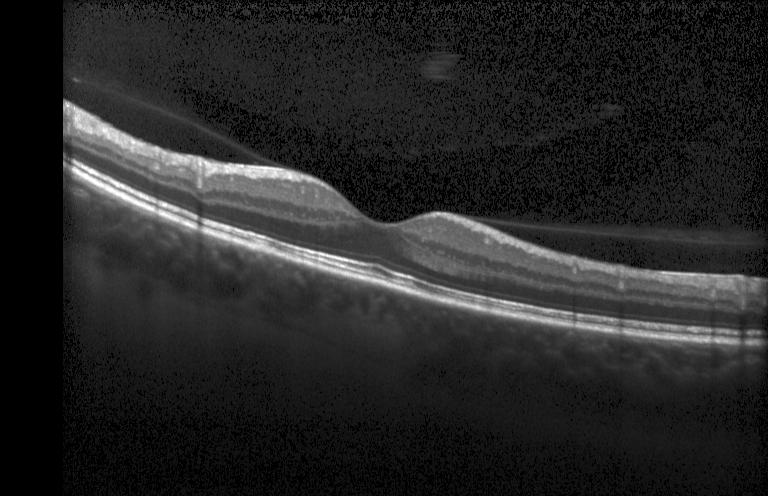 OCT line scan. SD-OCT
Macular OCT: neither choroidal neovascularization, diabetic macular edema, nor drusen.